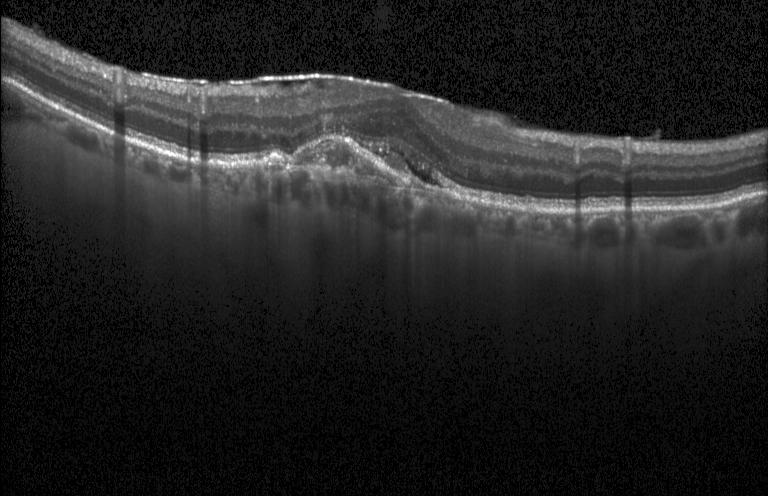 Instrument: Heidelberg Spectralis · fovea-centered · spectral-domain optical coherence tomography · OCT B-scan
Assessment: a choroidal neovascular membrane.